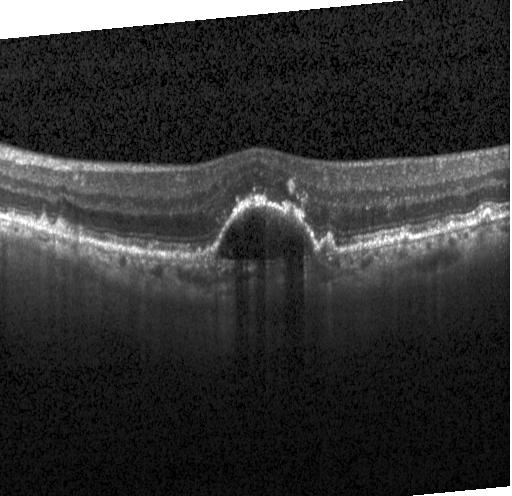

Finding: a choroidal neovascular membrane.